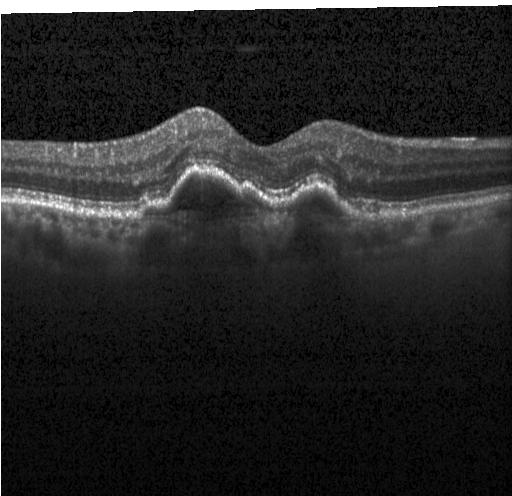

Retinal OCT B-scan.
Finding: a choroidal neovascular membrane.